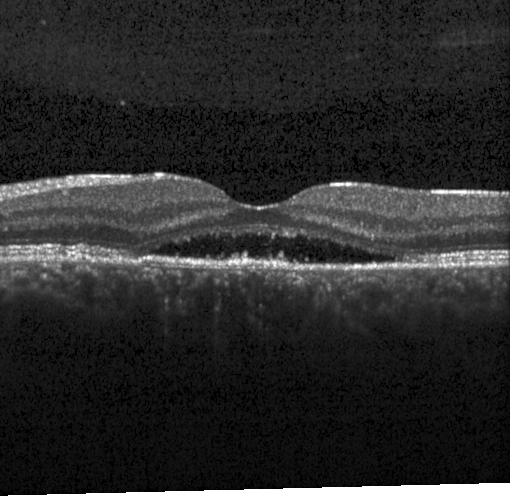 CNV.